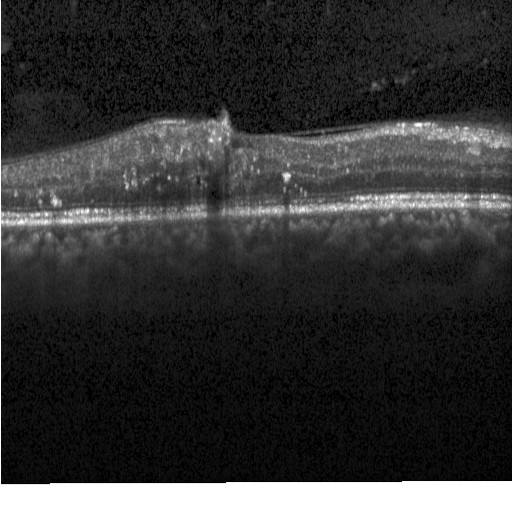 Dx: diabetic macular edema.